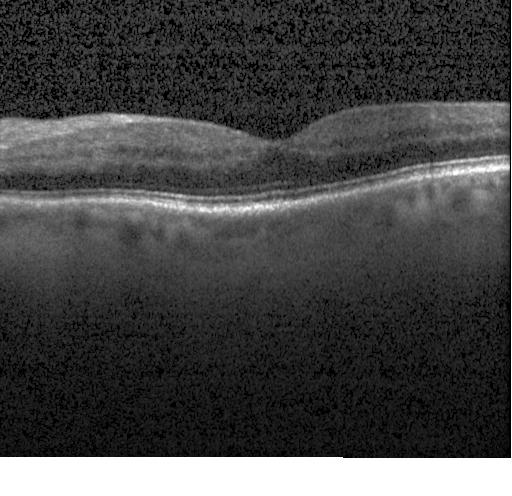

The scan shows neither choroidal neovascularization, diabetic macular edema, nor drusen.